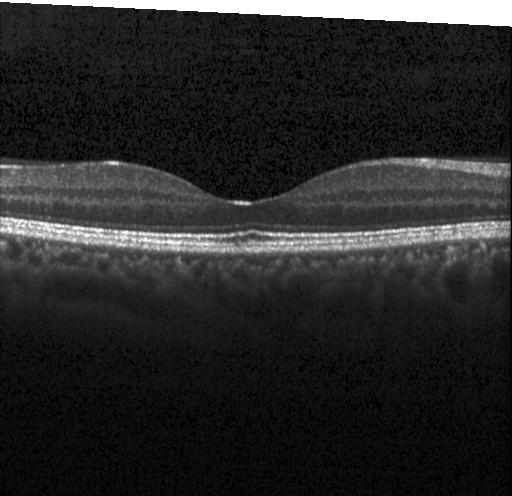 OCT line scan.
Impression: no choroidal neovascularization, diabetic macular edema, or drusen.